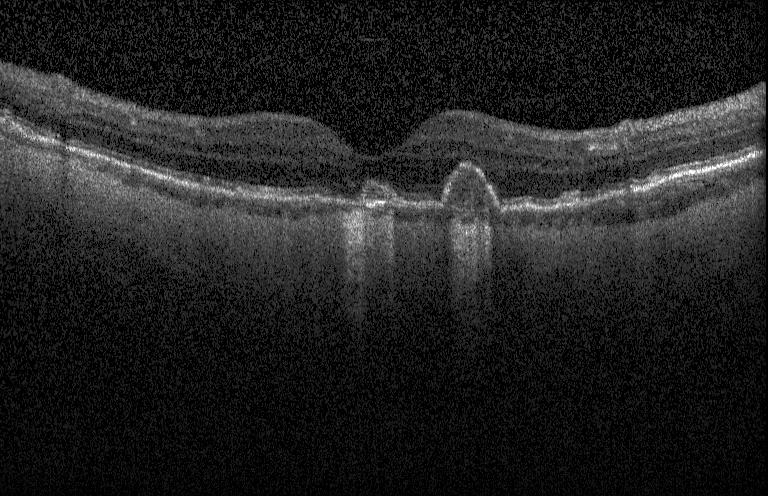 This B-scan demonstrates a choroidal neovascular membrane.